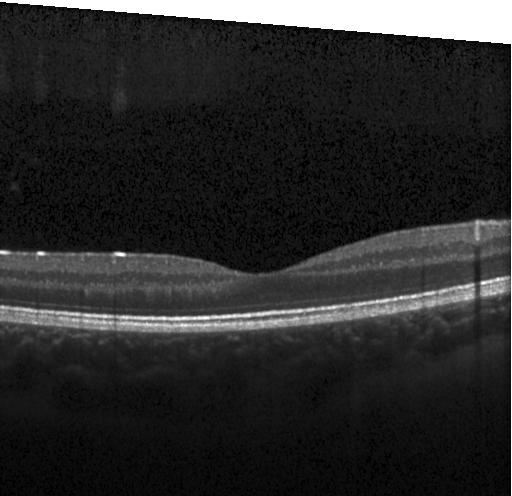 Impression: no CNV, no DME, and no drusen.